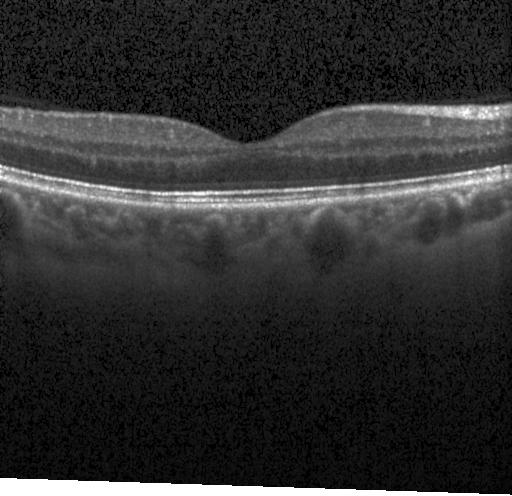

OCT line scan; instrument: Heidelberg Spectralis; spectral-domain OCT. Diagnosis: no evidence of choroidal neovascularization, diabetic macular edema, or drusen.